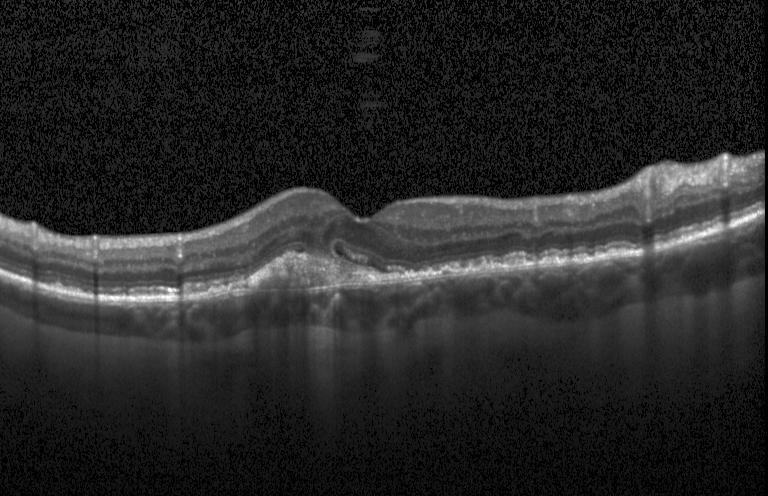

Optical coherence tomography B-scan
Diagnosis: a choroidal neovascular membrane.